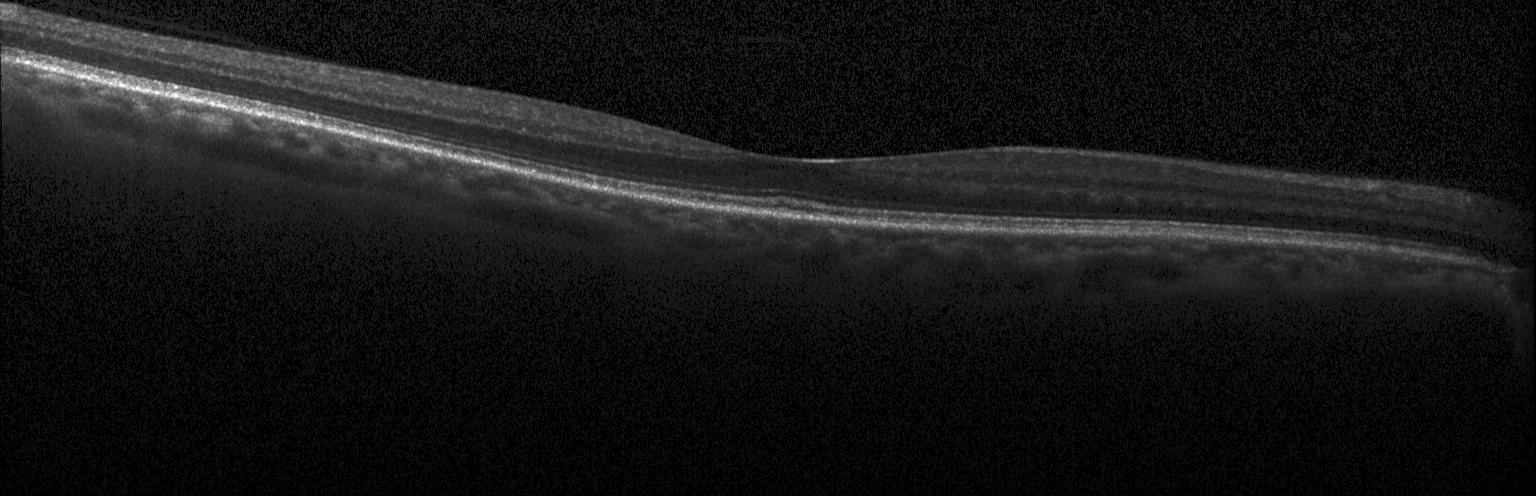

Optical coherence tomography scan; centered on the fovea. Finding: no choroidal neovascularization, diabetic macular edema, or drusen.